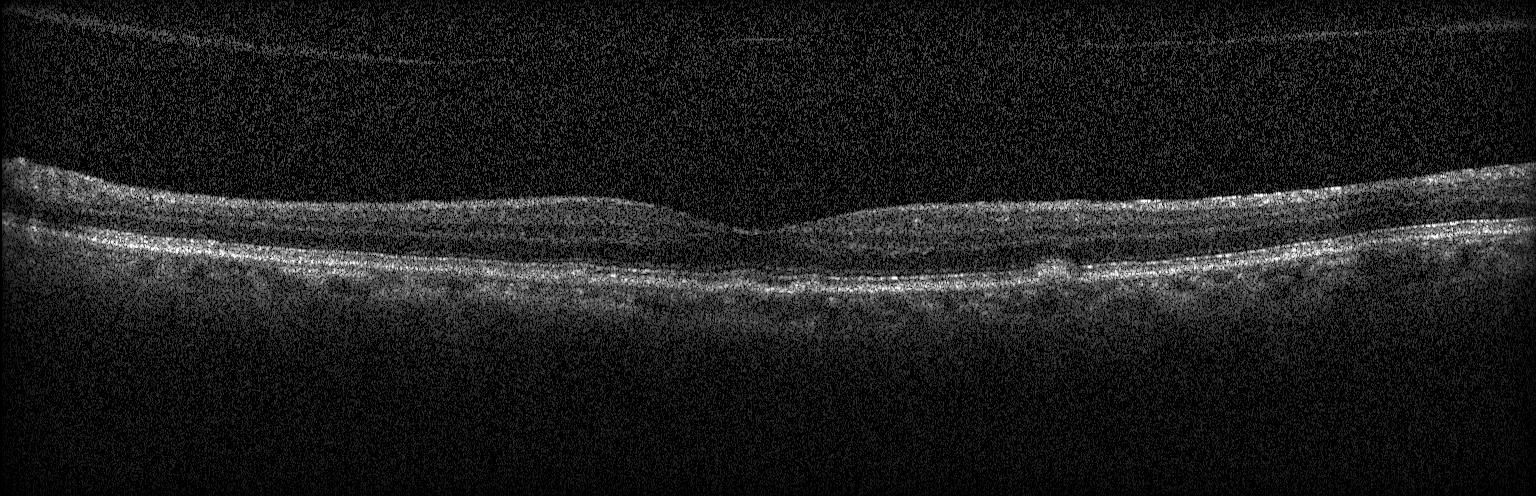 Optical coherence tomography B-scan. Finding: drusen.